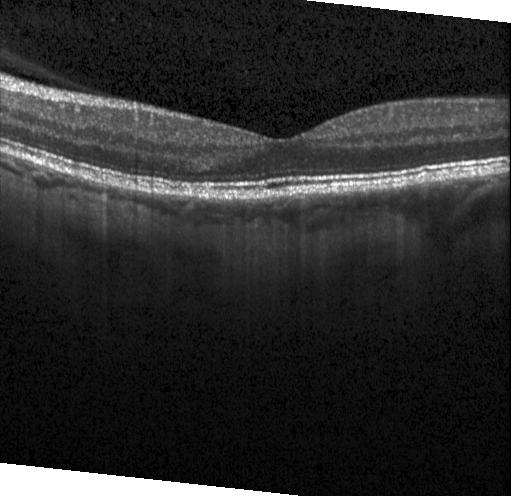
Finding: no evidence of choroidal neovascularization, diabetic macular edema, or drusen.